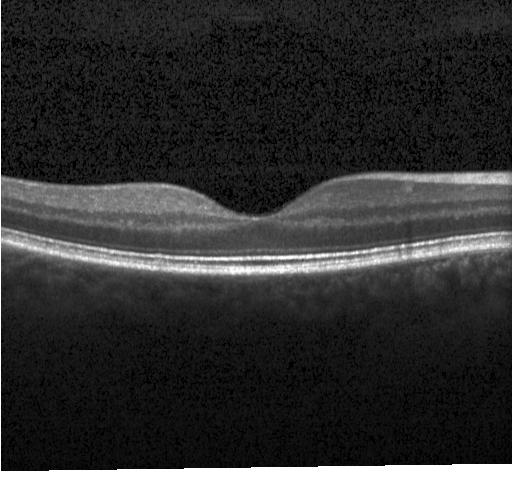 Diagnosis: neither CNV, DME, nor drusen.